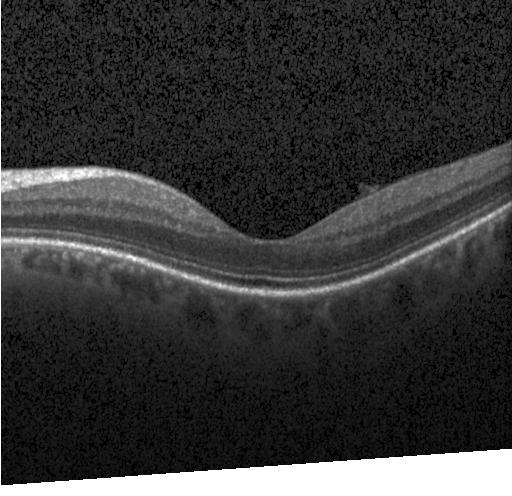 Impression: no choroidal neovascularization, diabetic macular edema, or drusen.